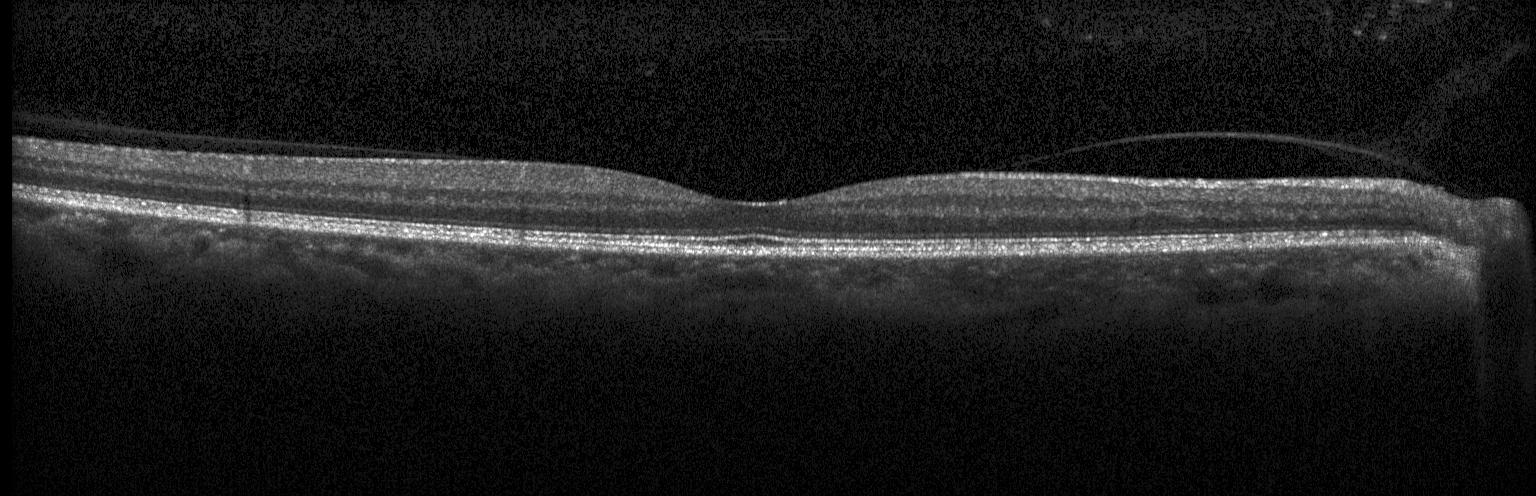

OCT B-scan — This B-scan demonstrates no choroidal neovascularization, diabetic macular edema, or drusen.